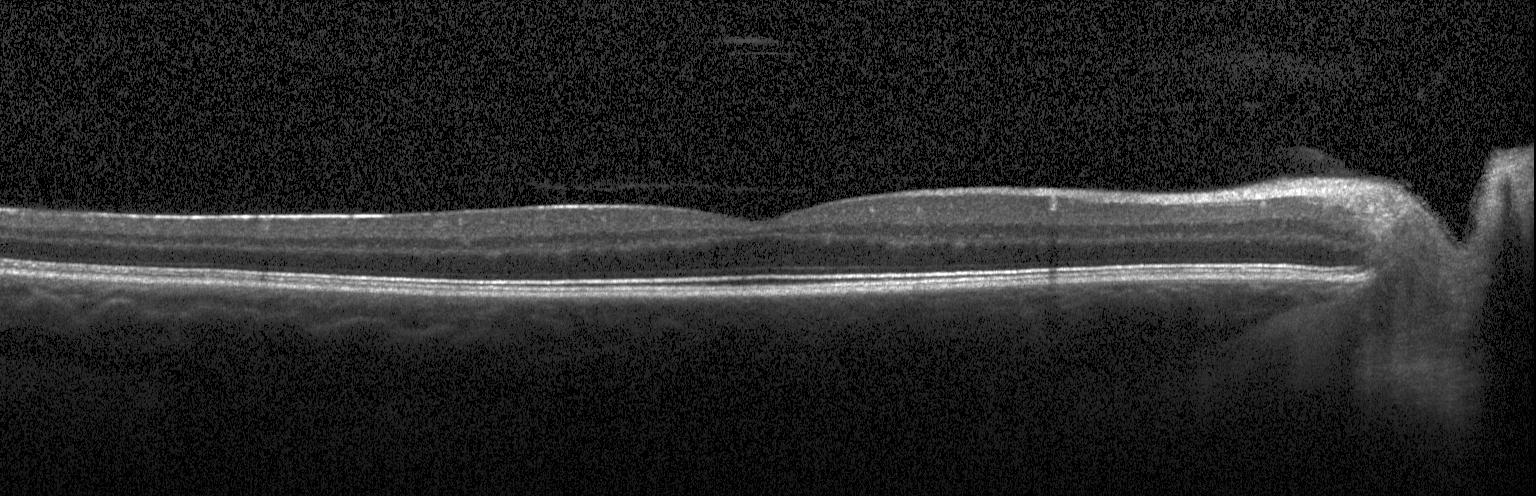
Retinal OCT cross-section showing no choroidal neovascularization, diabetic macular edema, or drusen.